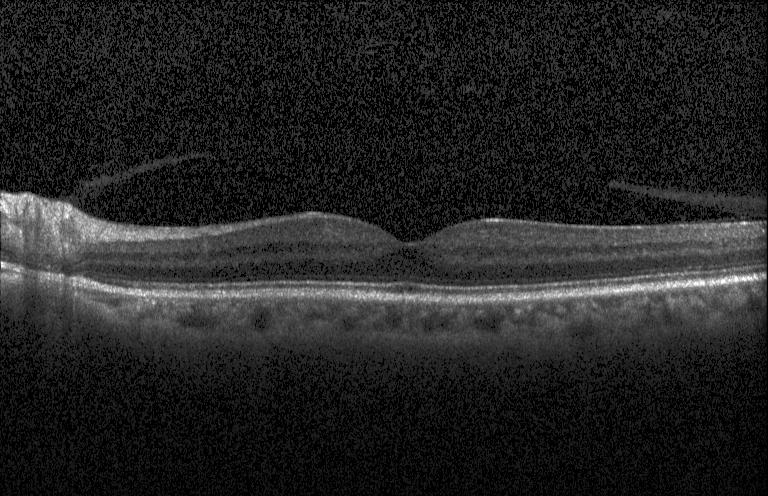 Retinal OCT cross-section — Impression: no choroidal neovascularization, diabetic macular edema, or drusen.